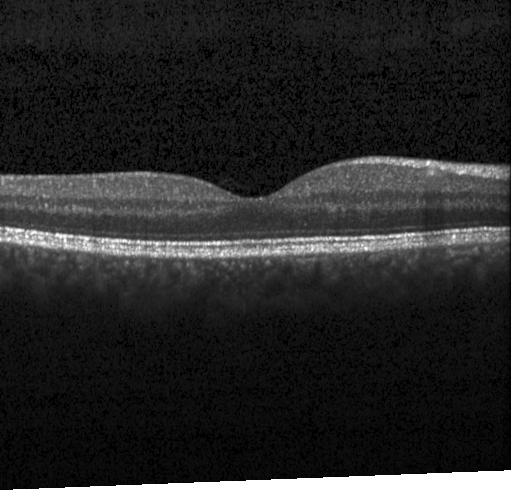 Retinal OCT cross-section — No evidence of choroidal neovascularization, diabetic macular edema, or drusen.